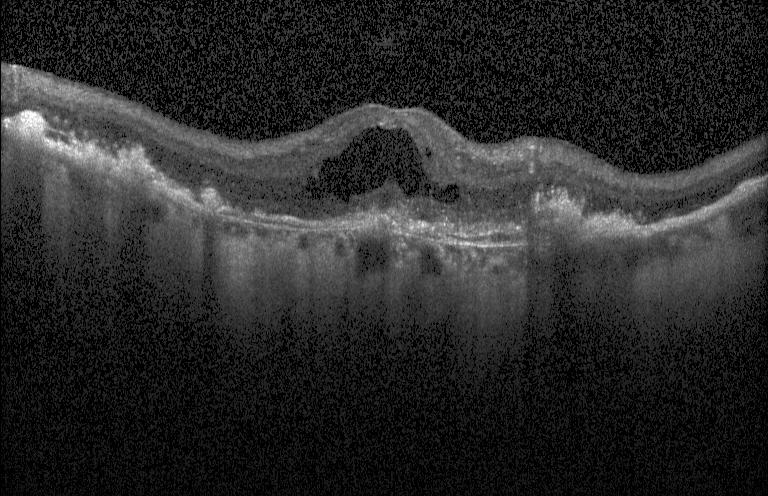

Heidelberg Spectralis, retinal OCT B-scan.
Impression: a choroidal neovascular membrane.